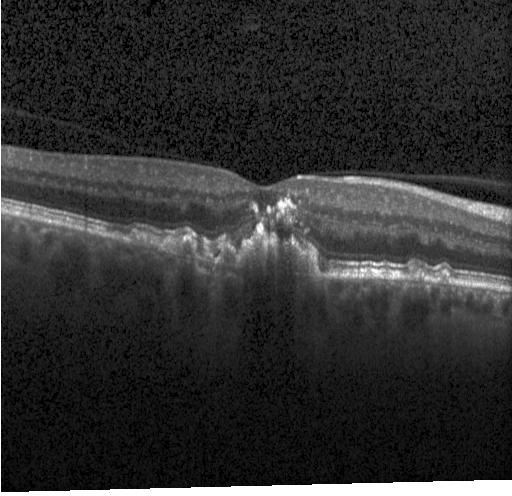 Spectral-domain OCT B-scan: choroidal neovascularization (CNV).